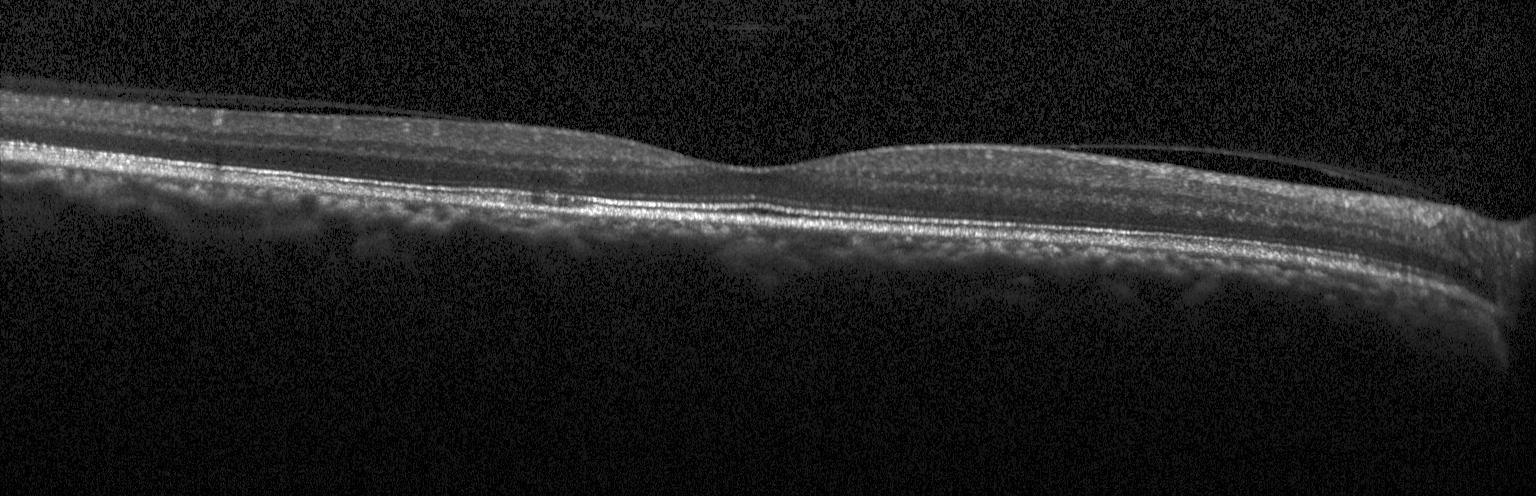

Heidelberg Spectralis OCT system, optical coherence tomography scan, SD-OCT
OCT finding: no evidence of CNV, DME, or drusen.